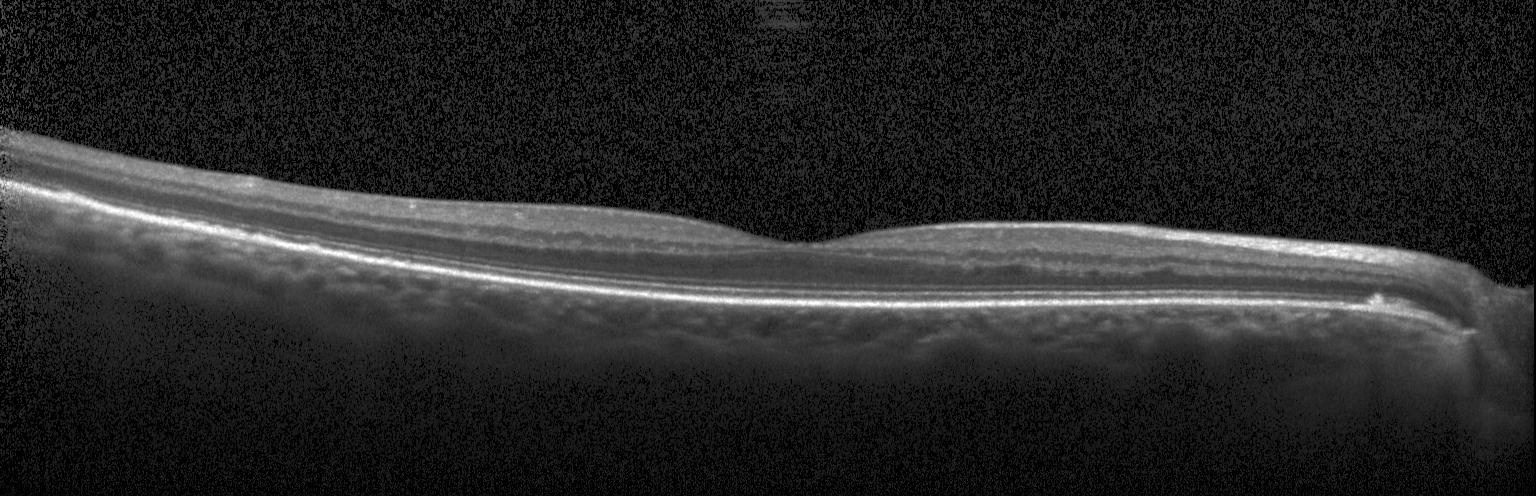 The scan shows neither choroidal neovascularization, diabetic macular edema, nor drusen.